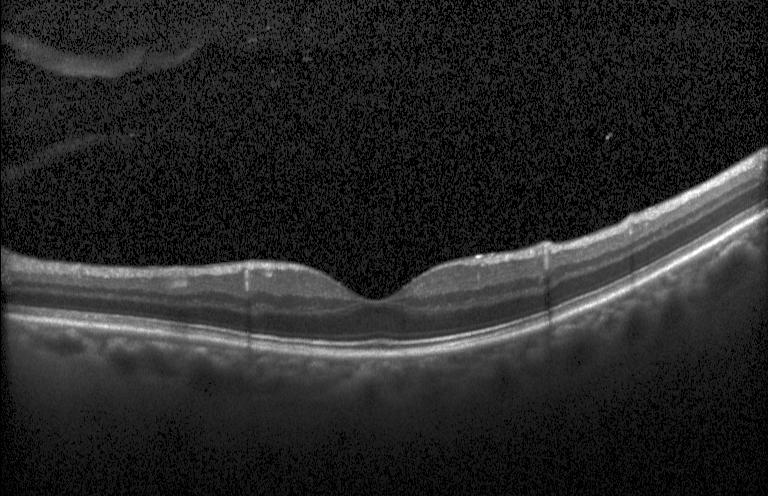

OCT B-scan
Diagnosis: no CNV, no DME, and no drusen.